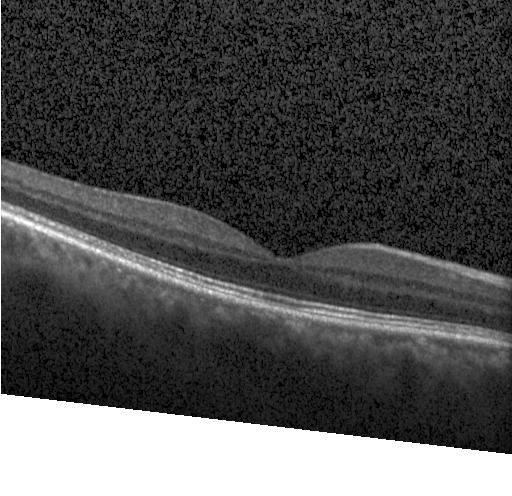 SD-OCT, optical coherence tomography B-scan
Macular OCT: no choroidal neovascularization, diabetic macular edema, or drusen.